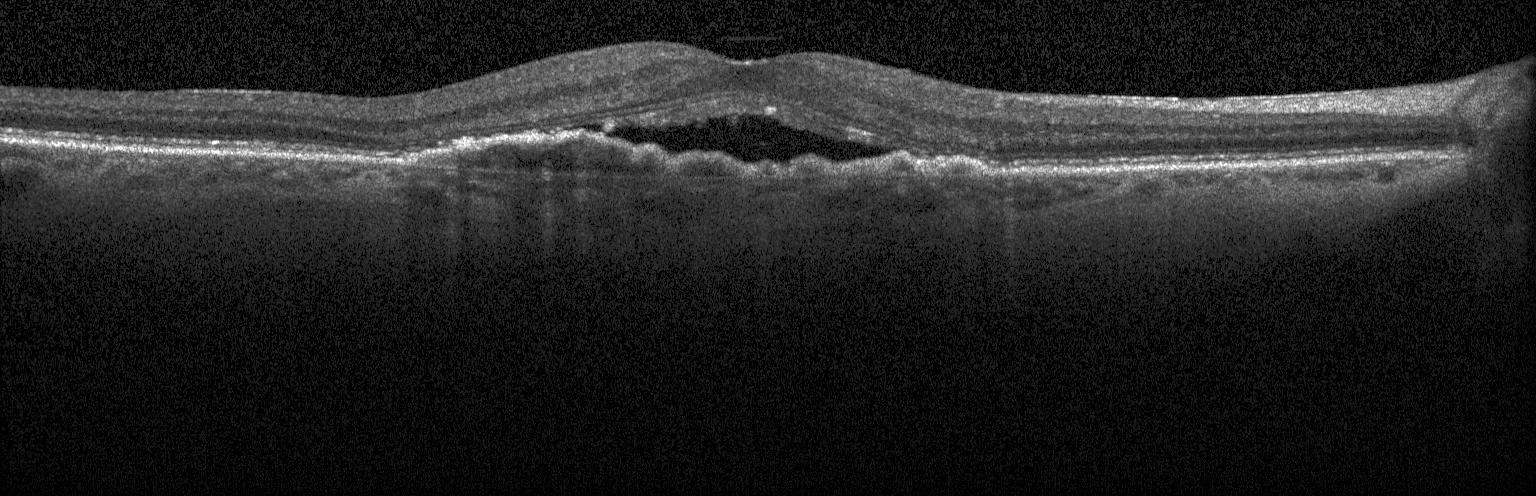

Macular scan, retinal OCT B-scan, instrument: Heidelberg Spectralis, SD-OCT.
Choroidal neovascularization (CNV).